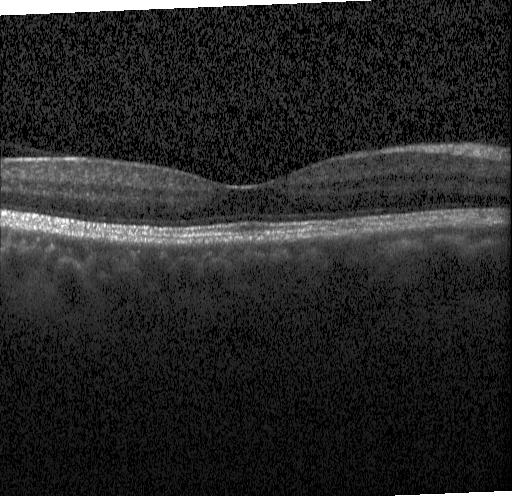
Fovea-centered; retinal OCT B-scan; SD-OCT — Macular OCT: no evidence of CNV, DME, or drusen.